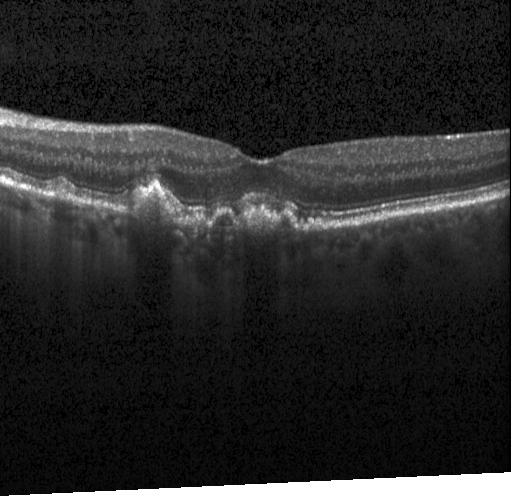

Diagnosis: choroidal neovascularization.